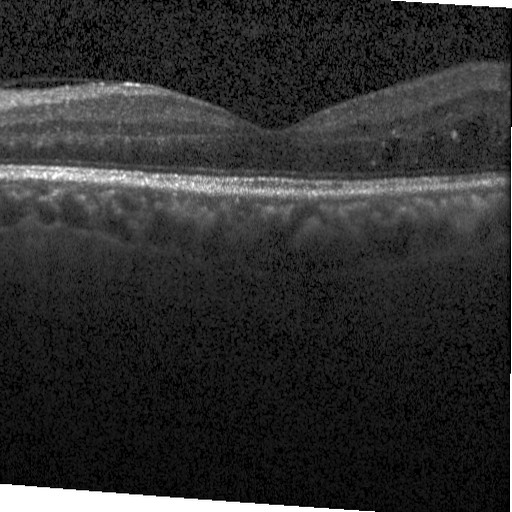

Spectral-domain OCT. Instrument: Heidelberg Spectralis. Retinal OCT B-scan. Horizontal scan through the fovea. Finding: DME.